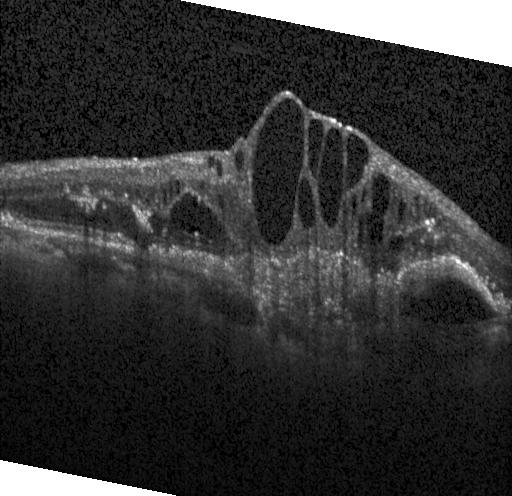 Macular scan; OCT line scan; SD-OCT
A choroidal neovascular membrane.